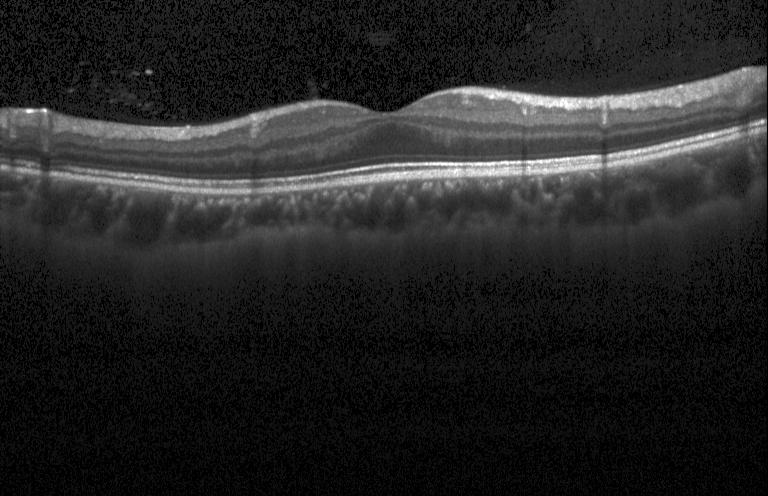

Diagnosis: no CNV, DME, or drusen.